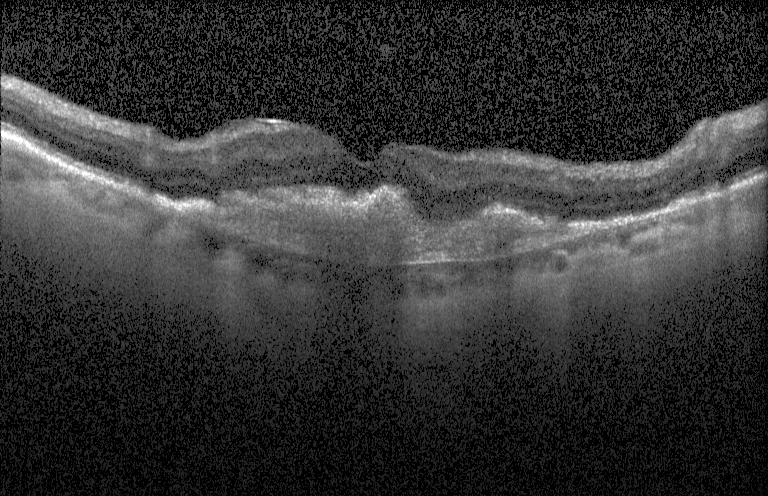
Heidelberg Spectralis, spectral-domain optical coherence tomography, macular scan, optical coherence tomography B-scan
Impression: choroidal neovascularization.